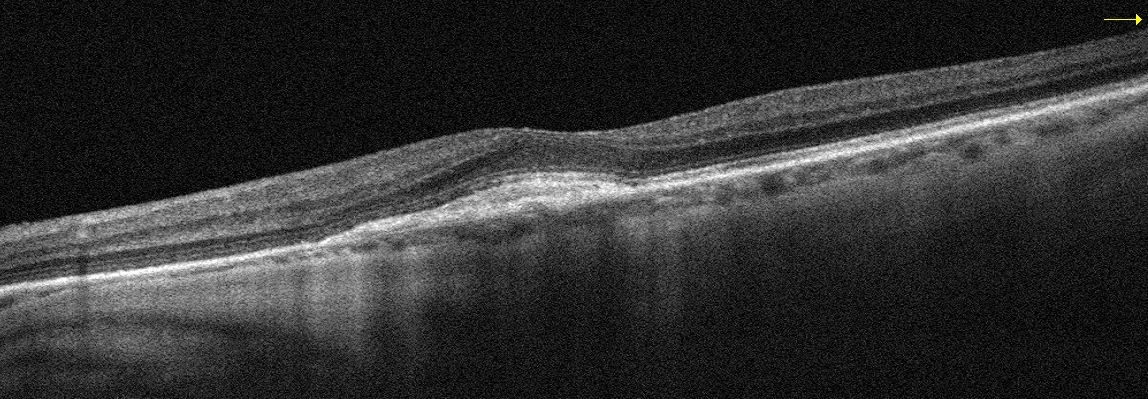

Optical coherence tomography B-scan; acquired on an Optovue Avanti RTVue XR — Finding: AMD.